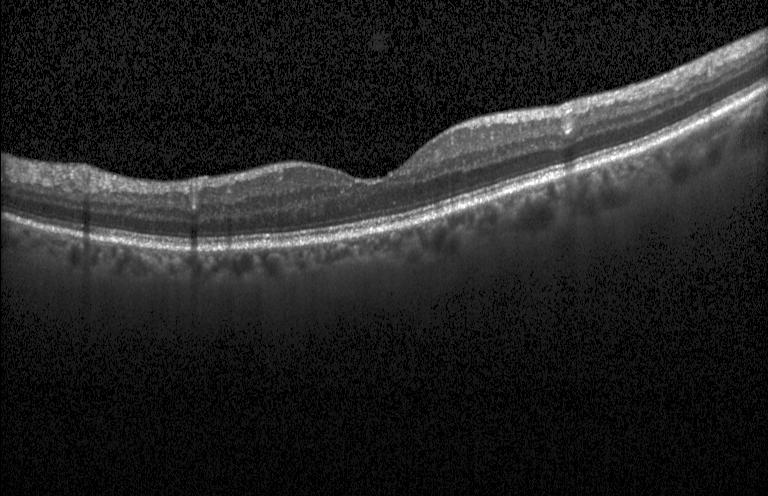 Acquired on a Heidelberg Spectralis; retinal OCT B-scan; spectral-domain optical coherence tomography — Finding: no evidence of CNV, DME, or drusen.